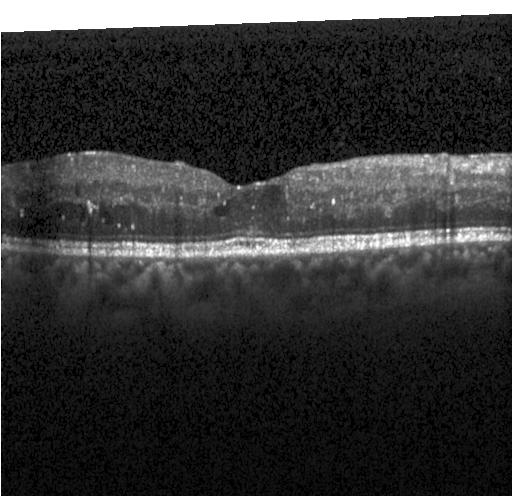

Retinal OCT cross-section. Assessment: diabetic macular edema.